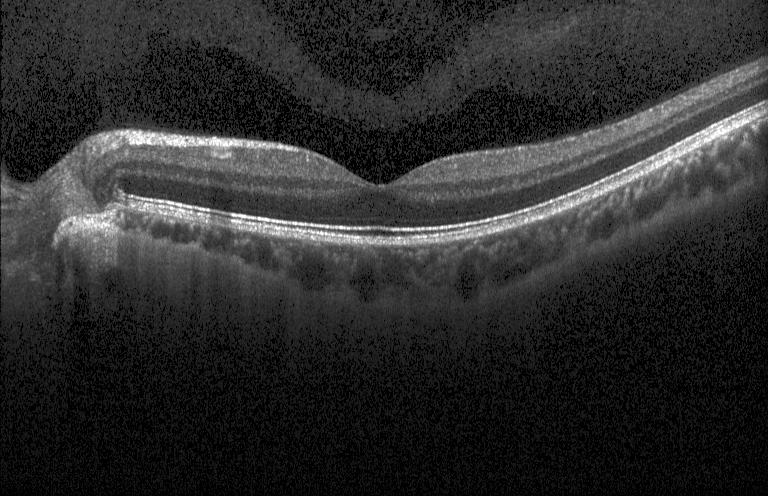 Instrument: Heidelberg Spectralis; spectral-domain OCT; OCT line scan. Finding: no choroidal neovascularization, no diabetic macular edema, and no drusen.